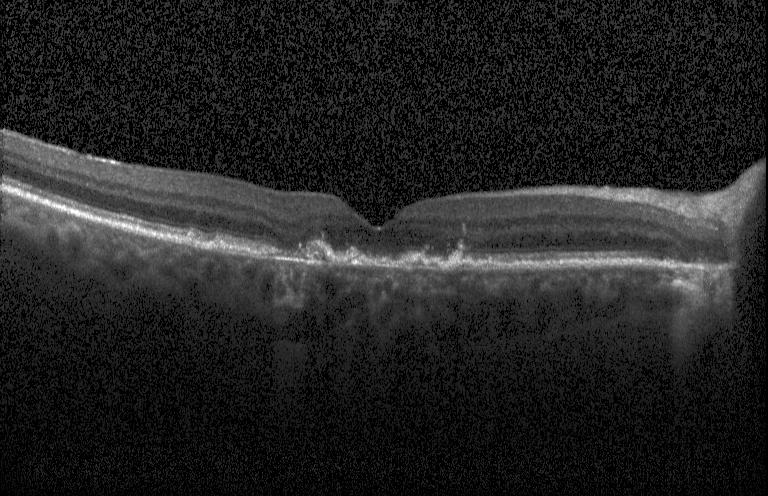
Retinal OCT B-scan — Diagnosis: choroidal neovascularization (CNV).